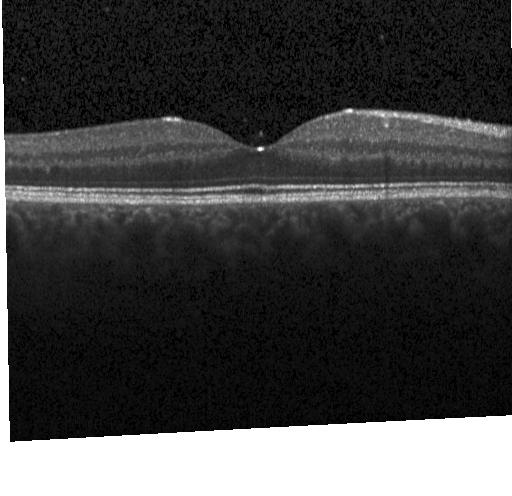 Optical coherence tomography B-scan — The scan shows no choroidal neovascularization, no diabetic macular edema, and no drusen.